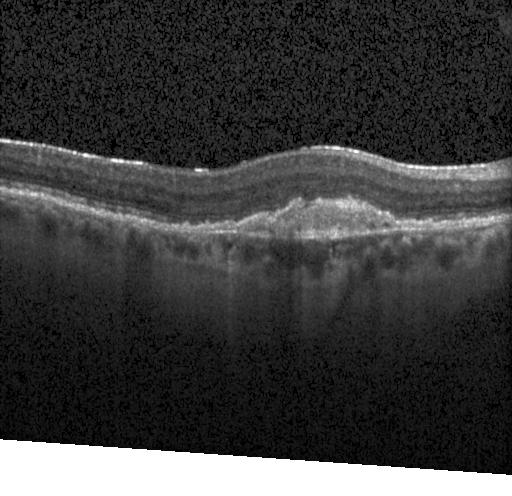

Impression: a choroidal neovascular membrane.